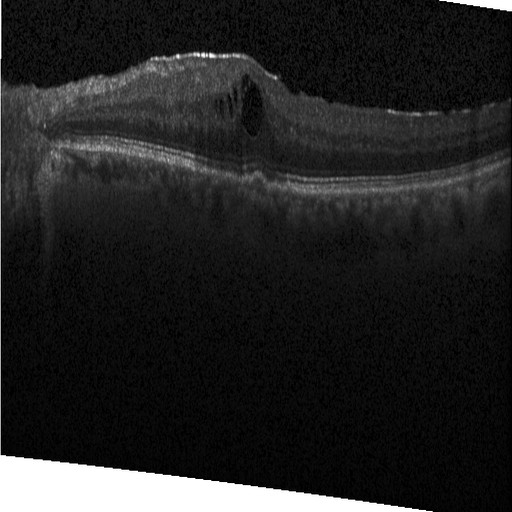

Optical coherence tomography scan.
Diagnosis: diabetic macular edema.